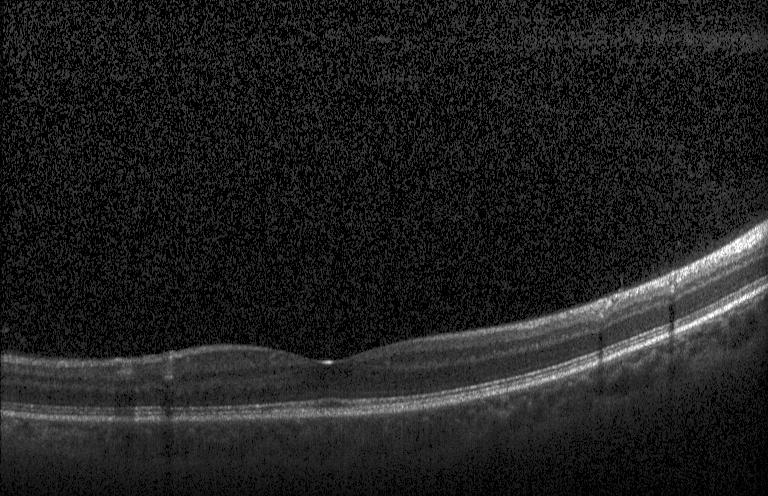

Spectral-domain OCT · centered on the fovea · OCT B-scan · acquired on a Heidelberg Spectralis. Impression: neither choroidal neovascularization, diabetic macular edema, nor drusen.